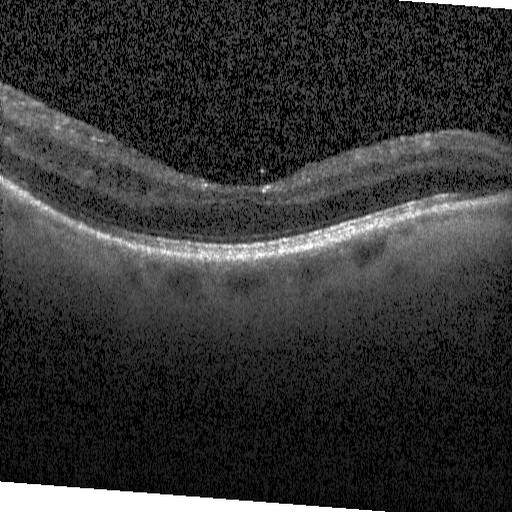
Macular scan · optical coherence tomography B-scan · acquired on a Heidelberg Spectralis. Dx: DME.